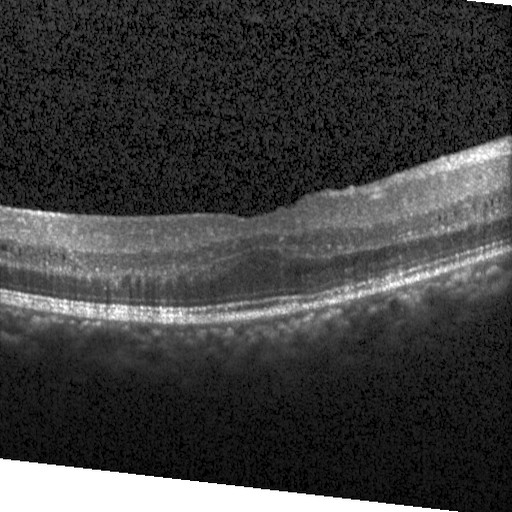

OCT finding: DME.